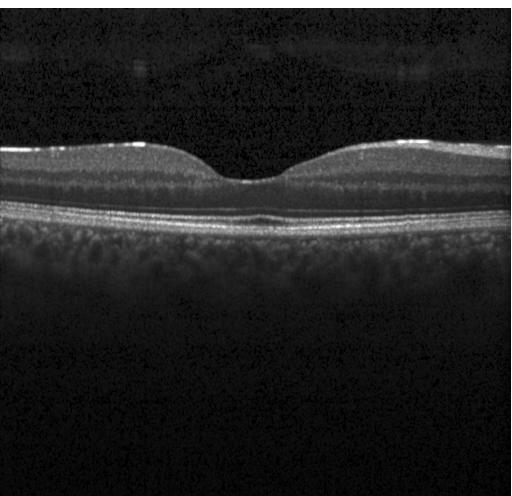

OCT line scan.
OCT finding: no choroidal neovascularization, no diabetic macular edema, and no drusen.